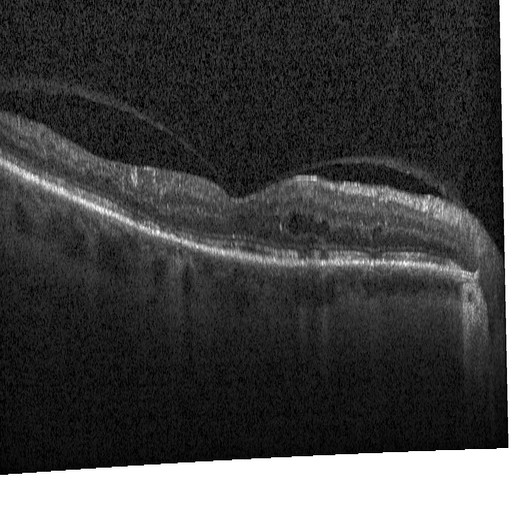 Finding: diabetic macular edema (DME).